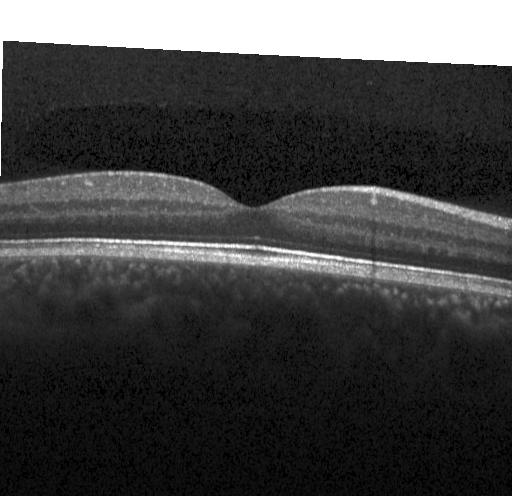 Assessment: no evidence of choroidal neovascularization, diabetic macular edema, or drusen.